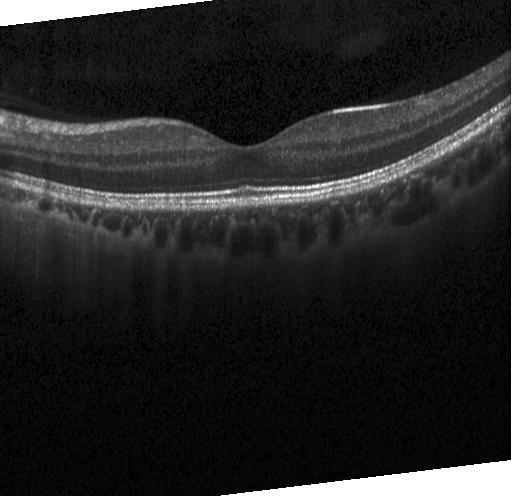

OCT line scan. Finding: neither choroidal neovascularization, diabetic macular edema, nor drusen.